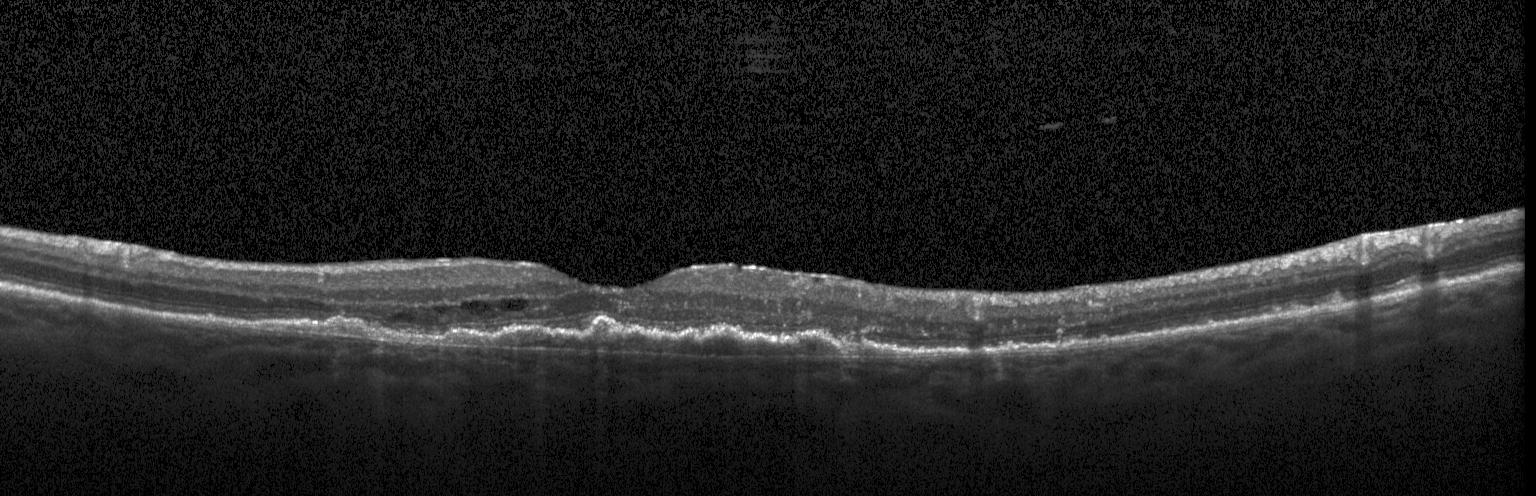 The scan shows choroidal neovascularization.